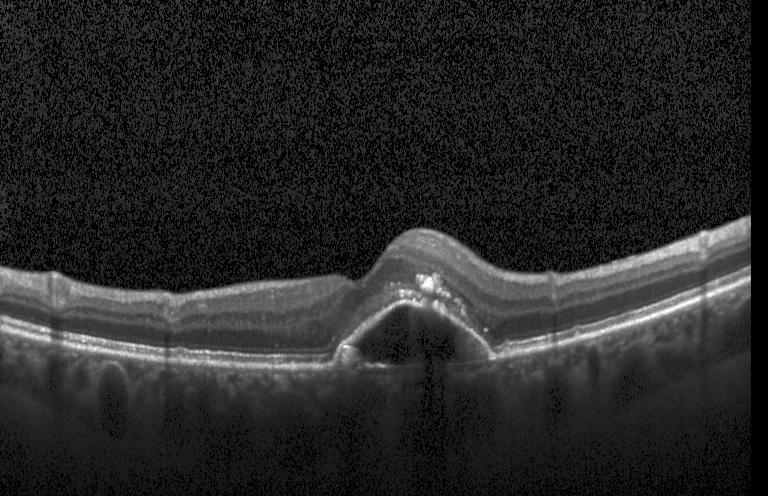

Retinal OCT B-scan. Impression: choroidal neovascularization (CNV).